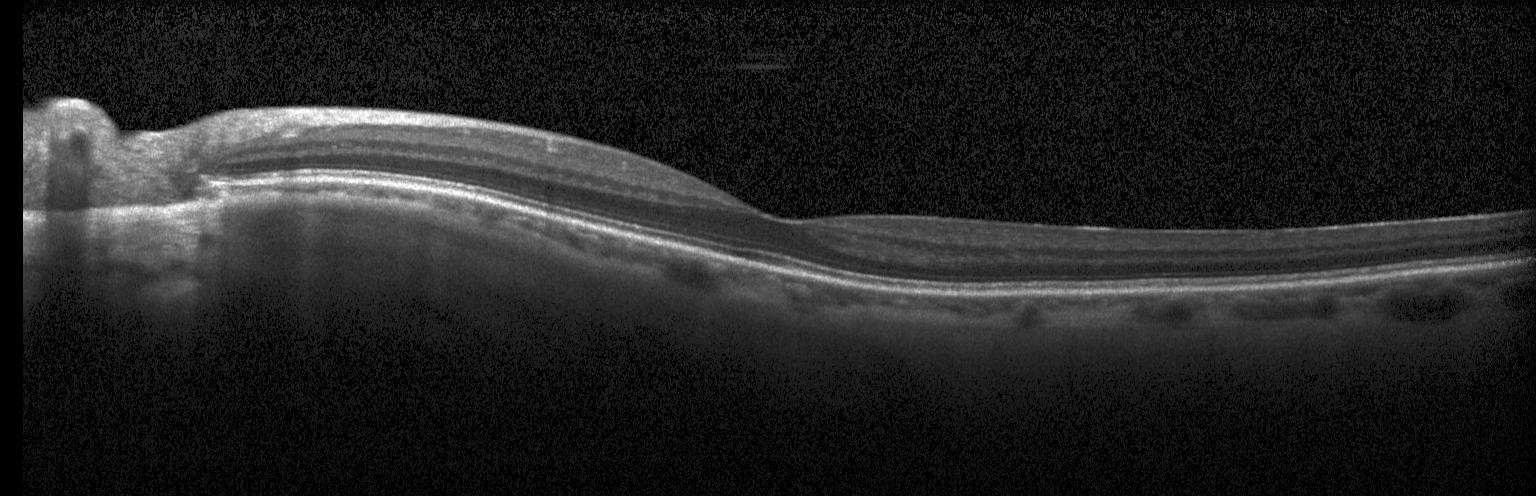

Macular OCT demonstrating no choroidal neovascularization, no diabetic macular edema, and no drusen.